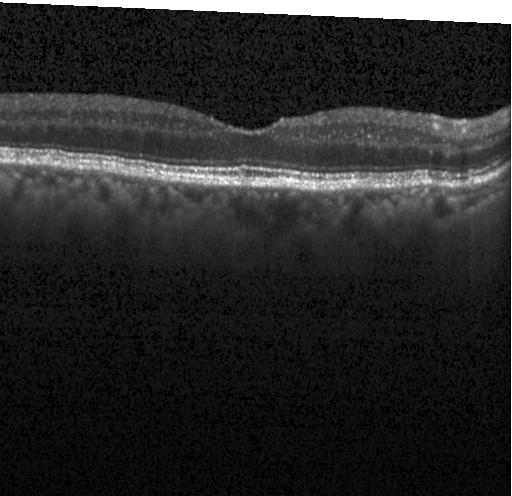
Retinal OCT cross-section, Heidelberg Spectralis.
Impression: no evidence of choroidal neovascularization, diabetic macular edema, or drusen.